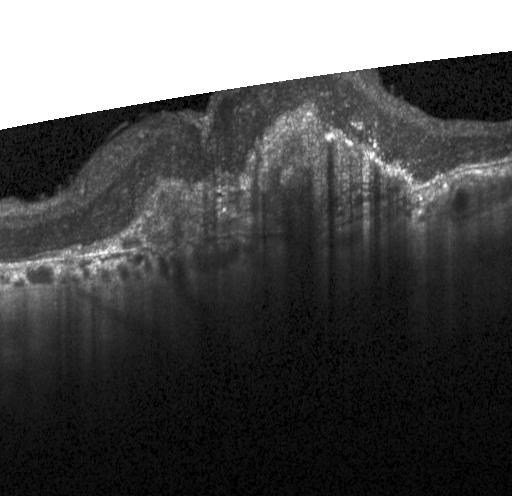

Retinal OCT cross-section showing CNV.